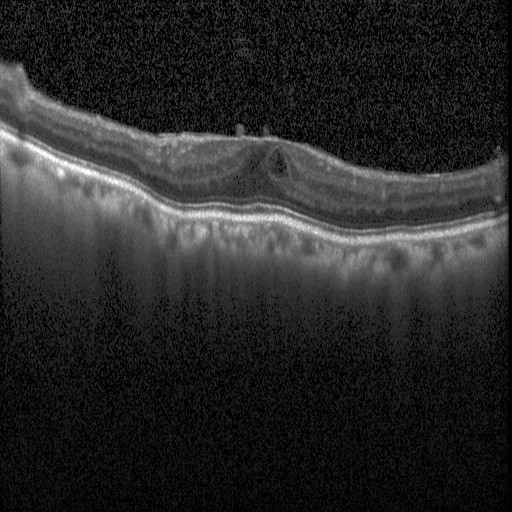
Macular OCT: diabetic macular edema (DME).